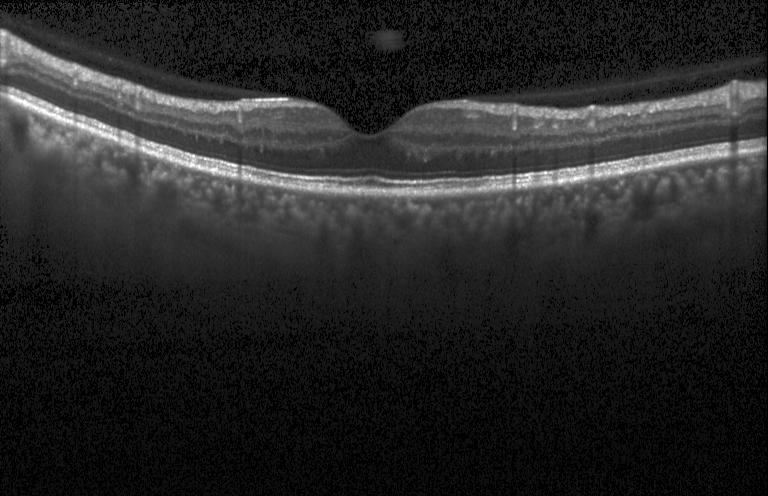 OCT finding: no choroidal neovascularization, diabetic macular edema, or drusen.